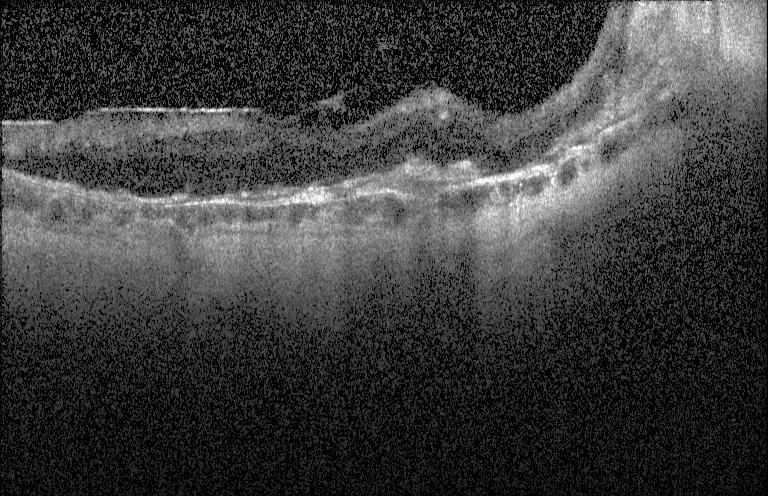
Optical coherence tomography scan, Heidelberg Spectralis OCT system
Impression: a choroidal neovascular membrane.